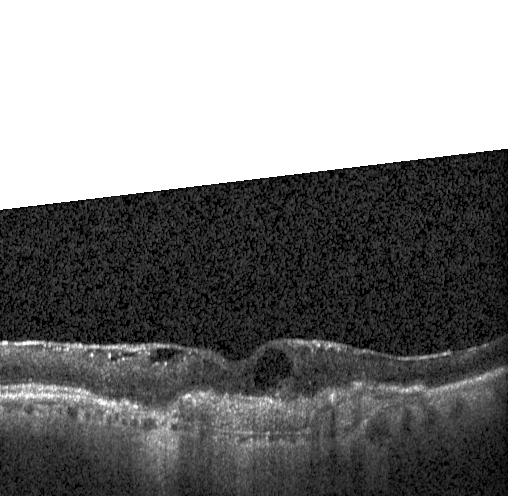
Retinal OCT B-scan. Acquired on a Heidelberg Spectralis. SD-OCT. Centered on the fovea — The scan shows a choroidal neovascular membrane.